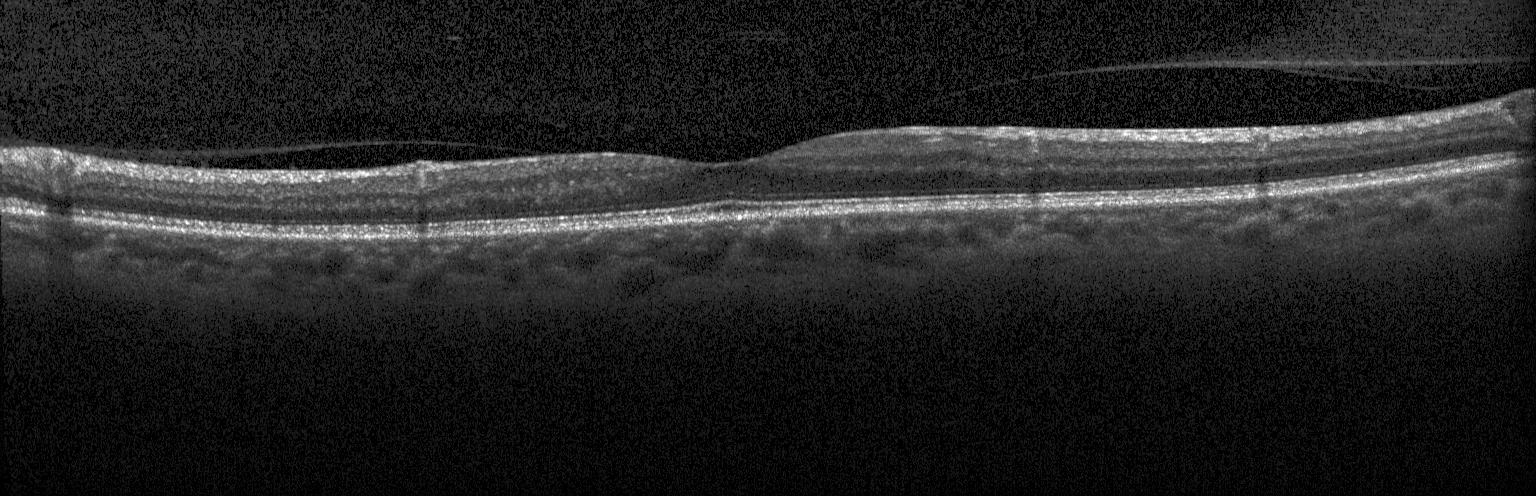 Optical coherence tomography scan · SD-OCT · horizontal scan through the fovea.
Finding: no evidence of choroidal neovascularization, diabetic macular edema, or drusen.